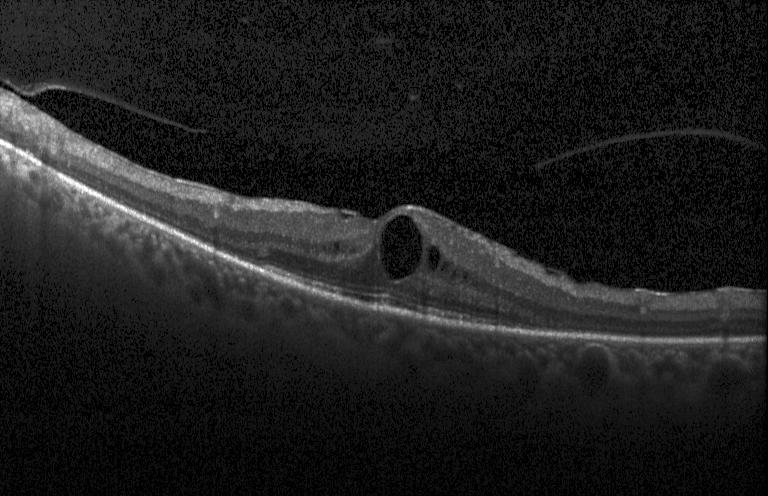
OCT B-scan. Spectral-domain OCT. Acquired on a Heidelberg Spectralis. The scan shows diabetic macular edema (DME).